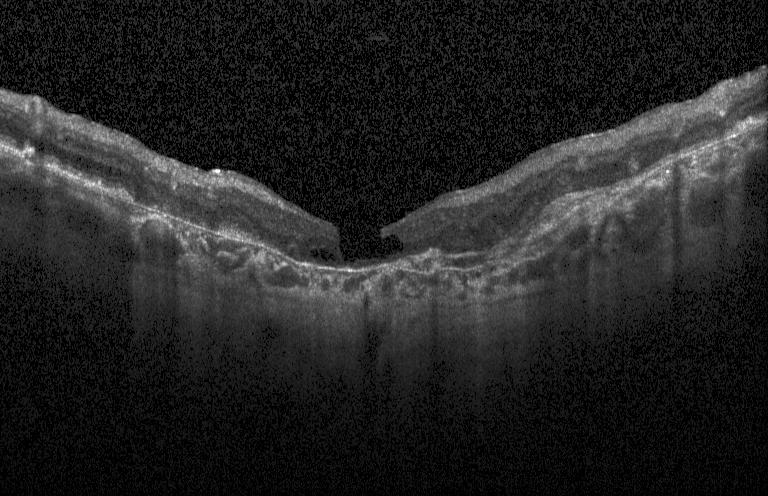
OCT B-scan.
Macular OCT: choroidal neovascularization (CNV).